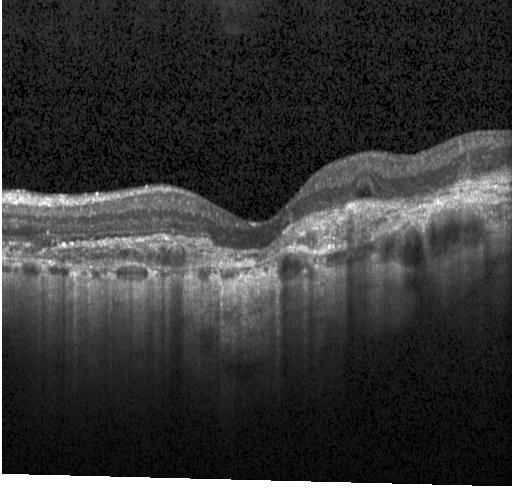
Instrument: Heidelberg Spectralis, optical coherence tomography scan — The scan shows a choroidal neovascular membrane.